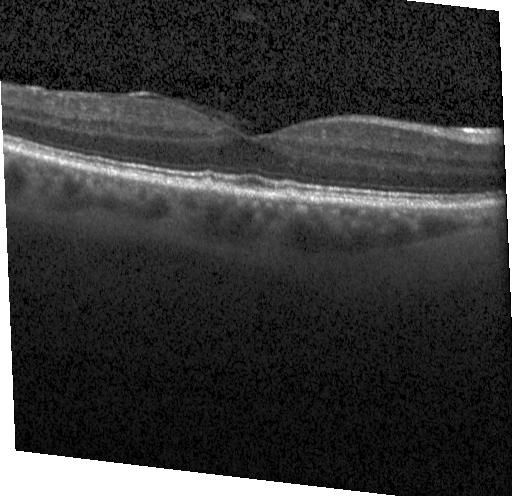
SD-OCT, retinal OCT cross-section, Heidelberg Spectralis
Finding: sub-RPE drusenoid deposits.